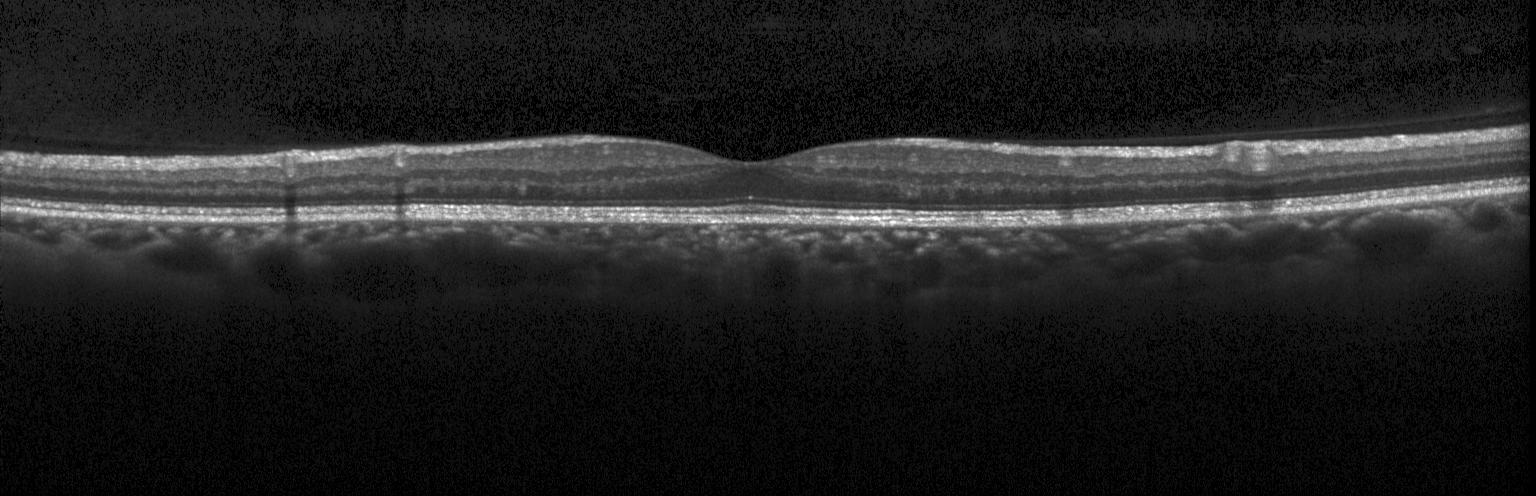 Diagnosis: no CNV, DME, or drusen.